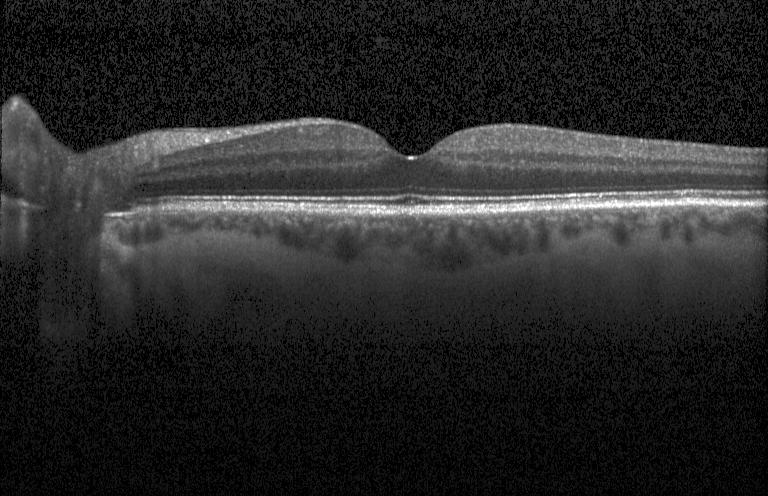

Retinal OCT B-scan; through the macula; spectral-domain optical coherence tomography; acquired on a Heidelberg Spectralis — Macular OCT: no choroidal neovascularization, diabetic macular edema, or drusen.